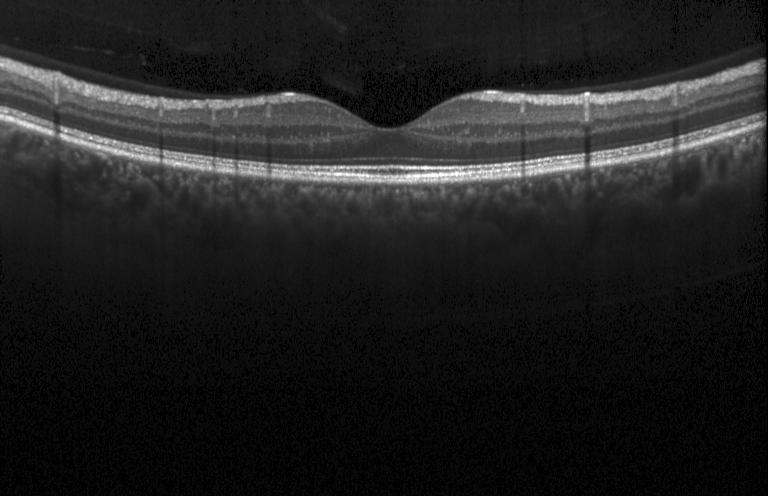 OCT line scan. Instrument: Heidelberg Spectralis. Fovea-centered. This B-scan demonstrates no choroidal neovascularization, no diabetic macular edema, and no drusen.